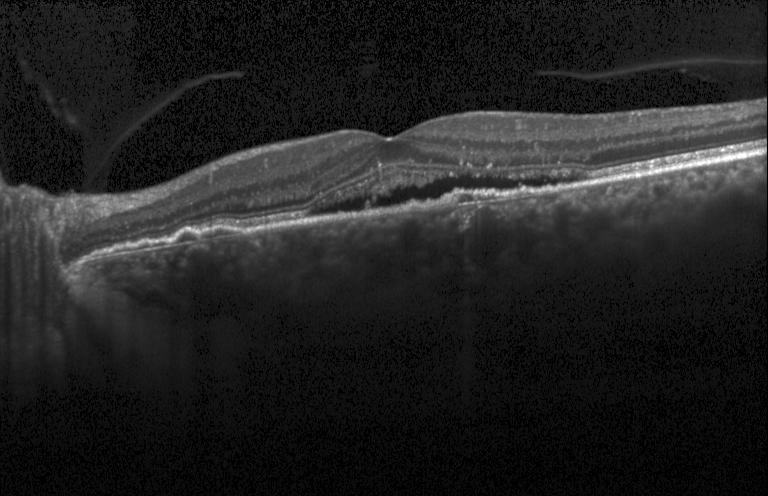

OCT line scan.
Choroidal neovascularization (CNV).